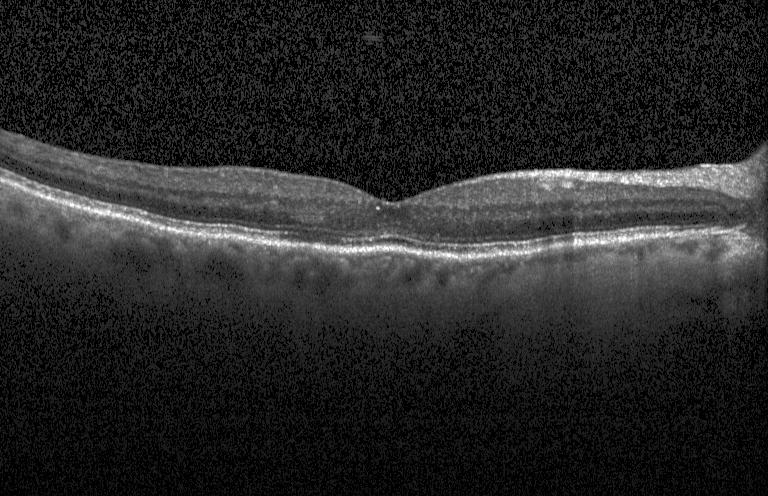

The scan shows no evidence of choroidal neovascularization, diabetic macular edema, or drusen.